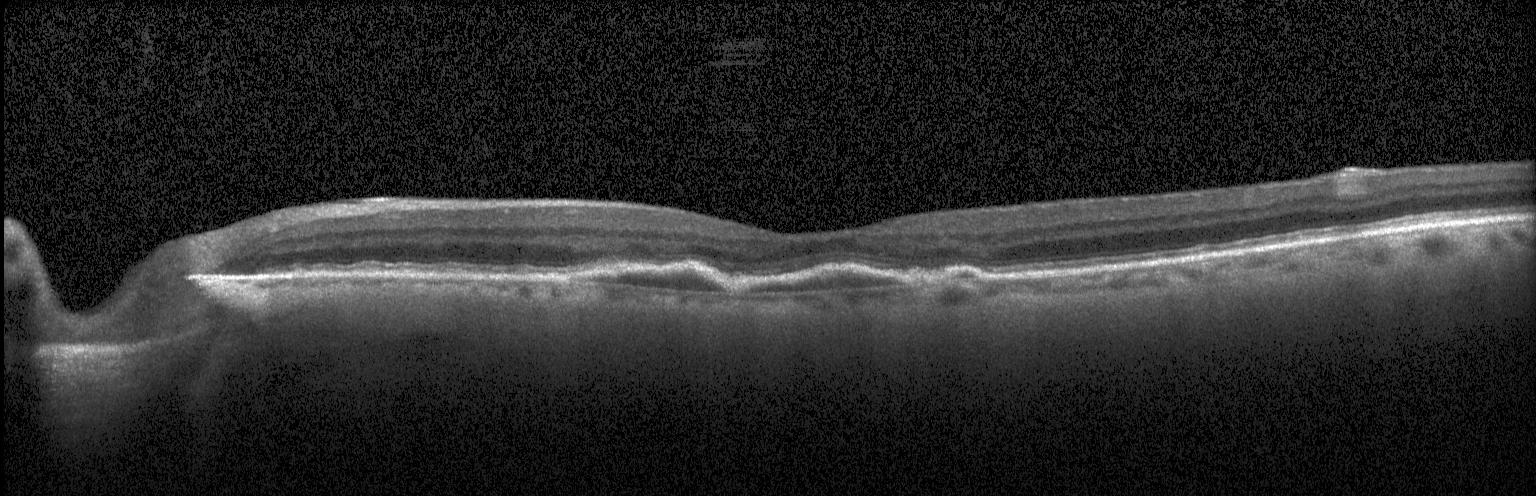
Macular OCT: a choroidal neovascular membrane.